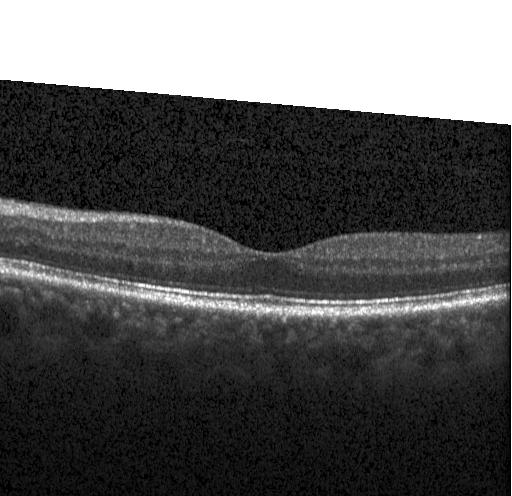

OCT finding: no choroidal neovascularization, no diabetic macular edema, and no drusen.